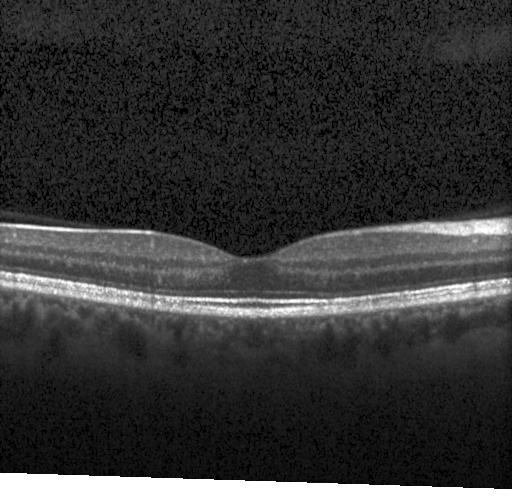
Optical coherence tomography B-scan
Finding: neither choroidal neovascularization, diabetic macular edema, nor drusen.